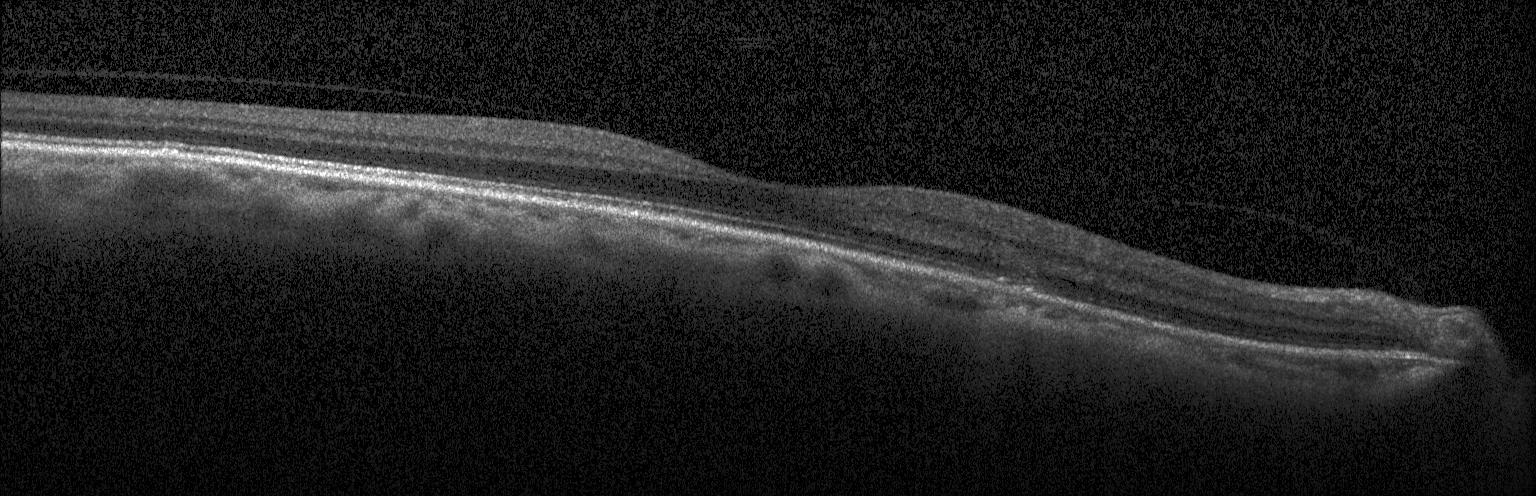
Macular OCT: neither choroidal neovascularization, diabetic macular edema, nor drusen.